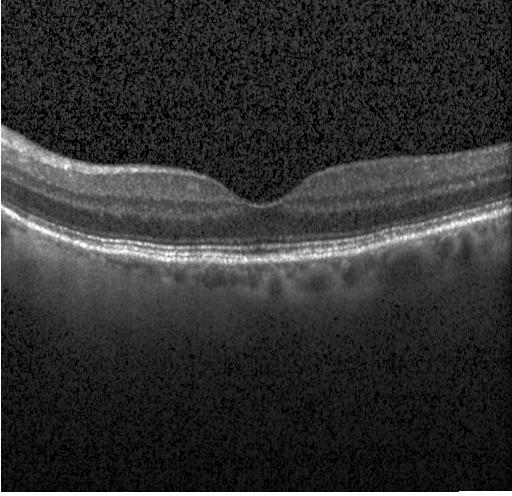 Macular OCT: no evidence of CNV, DME, or drusen.